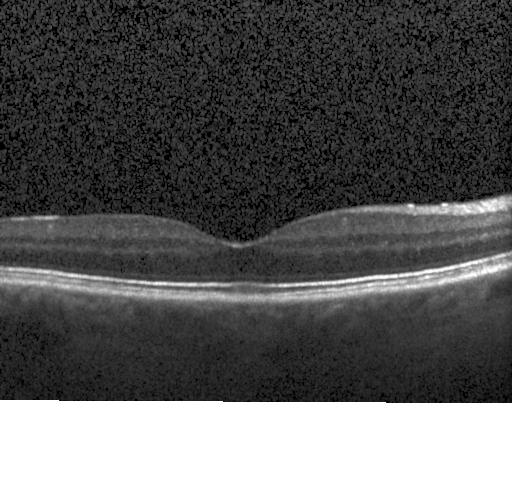 Retinal OCT B-scan; spectral-domain OCT; macular scan. Dx: neither choroidal neovascularization, diabetic macular edema, nor drusen.